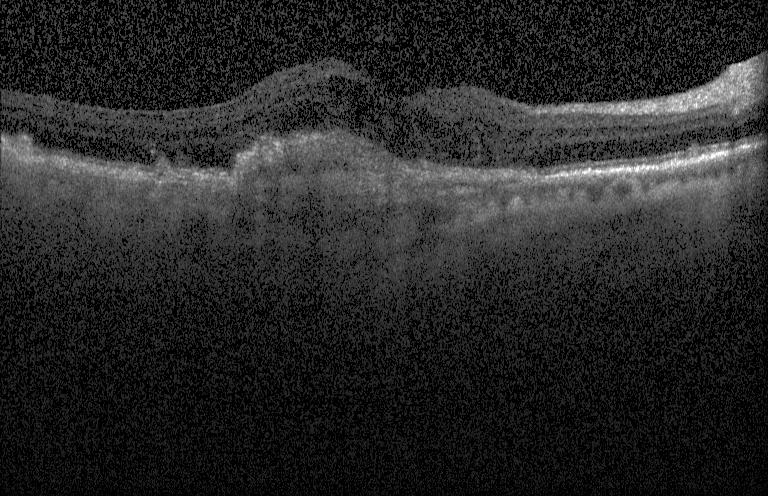

Diagnosis: a choroidal neovascular membrane.